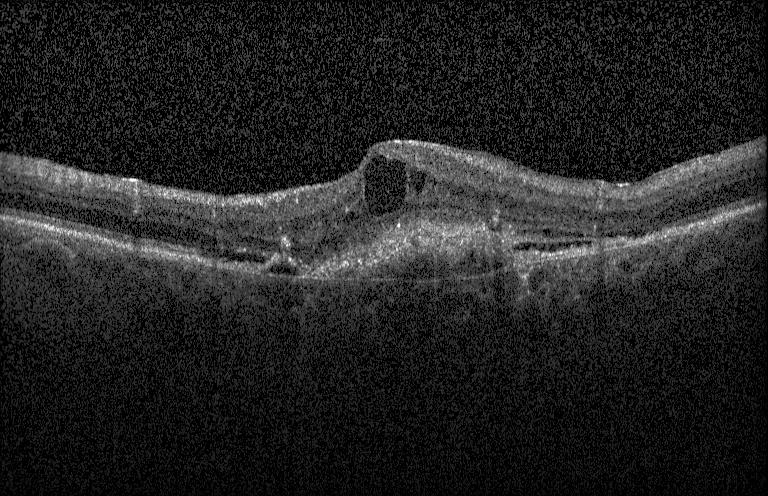
OCT B-scan showing choroidal neovascularization.